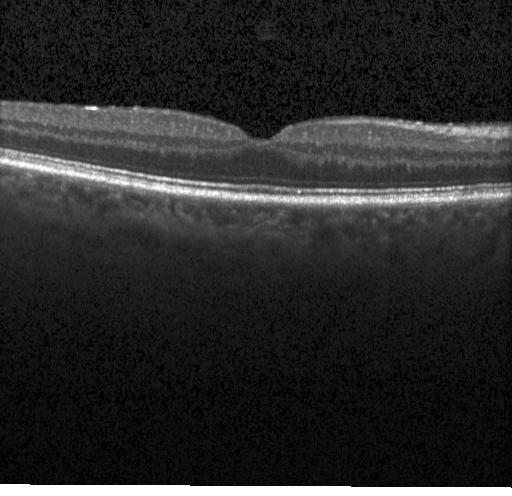

Retinal OCT B-scan.
Finding: no CNV, DME, or drusen.